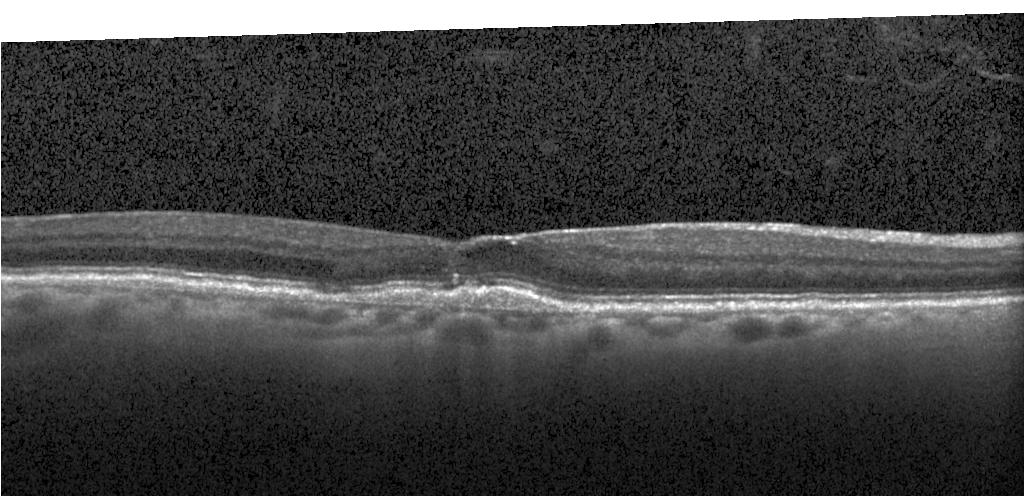 A choroidal neovascular membrane.